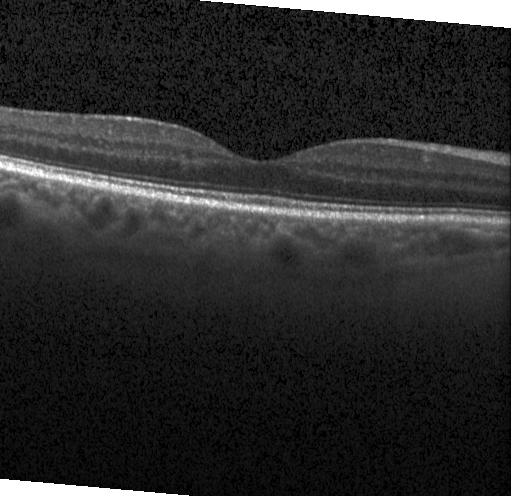

OCT B-scan. Spectral-domain OCT. Heidelberg Spectralis OCT system. Through the macula — Impression: neither choroidal neovascularization, diabetic macular edema, nor drusen.